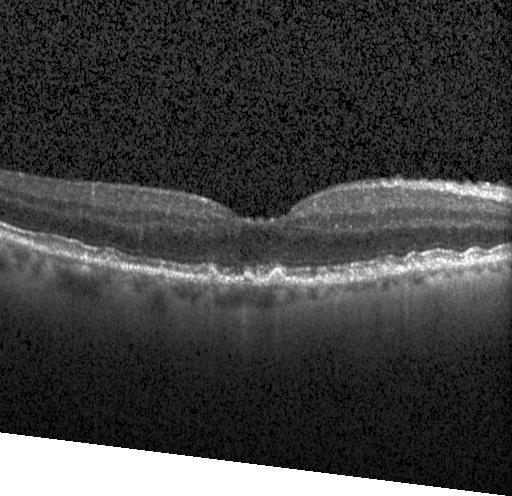

Diagnosis: sub-RPE drusenoid deposits.